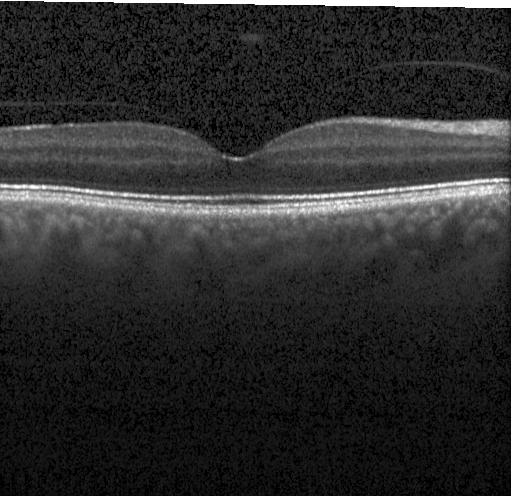

Heidelberg Spectralis. Optical coherence tomography scan.
Dx: no choroidal neovascularization, no diabetic macular edema, and no drusen.